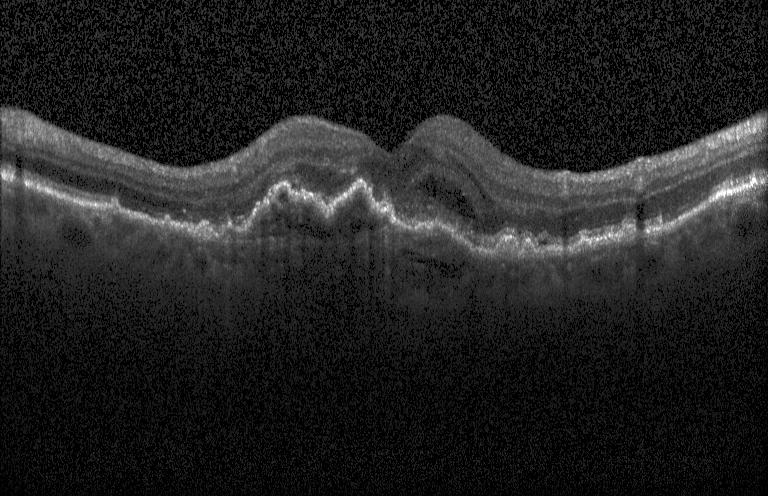 Acquired on a Heidelberg Spectralis, OCT B-scan, spectral-domain OCT, horizontal scan through the fovea. Diagnosis: a choroidal neovascular membrane.